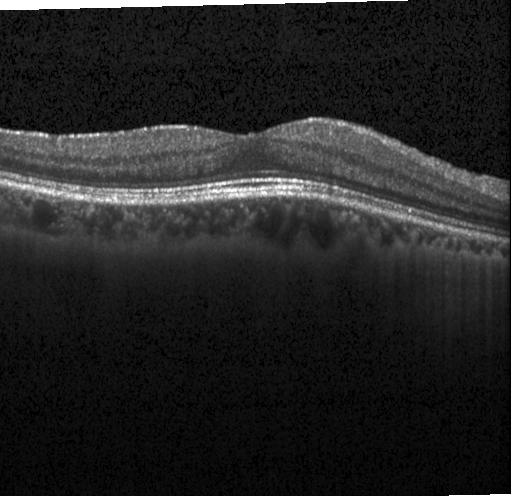 OCT finding: neither choroidal neovascularization, diabetic macular edema, nor drusen.